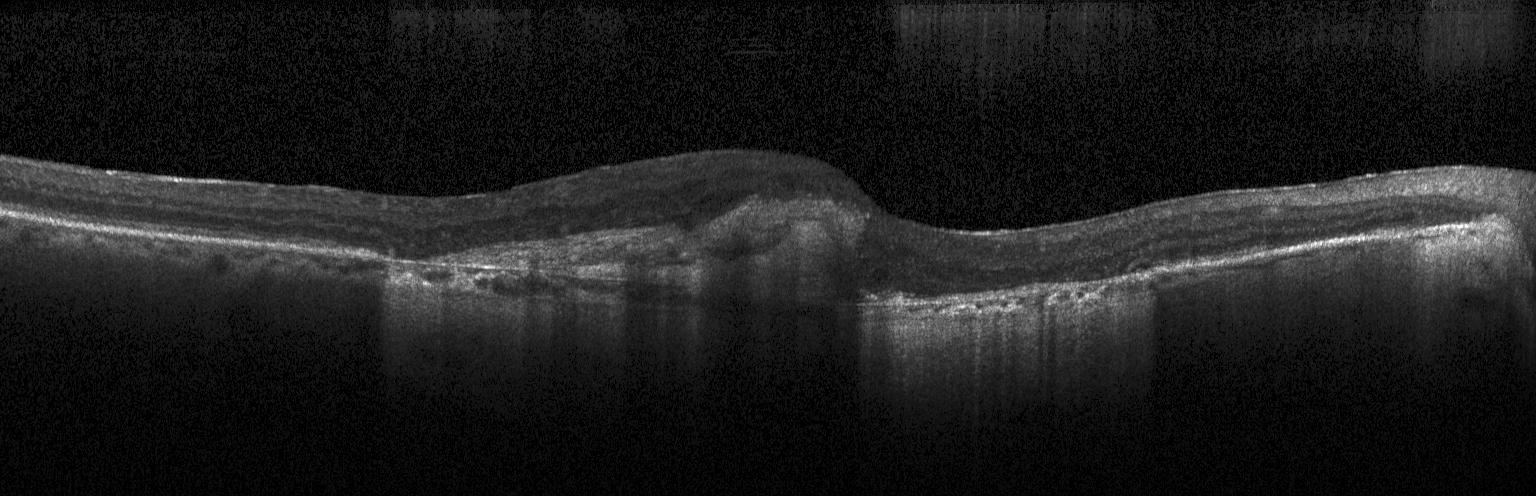

Spectral-domain optical coherence tomography; OCT line scan
OCT finding: CNV.